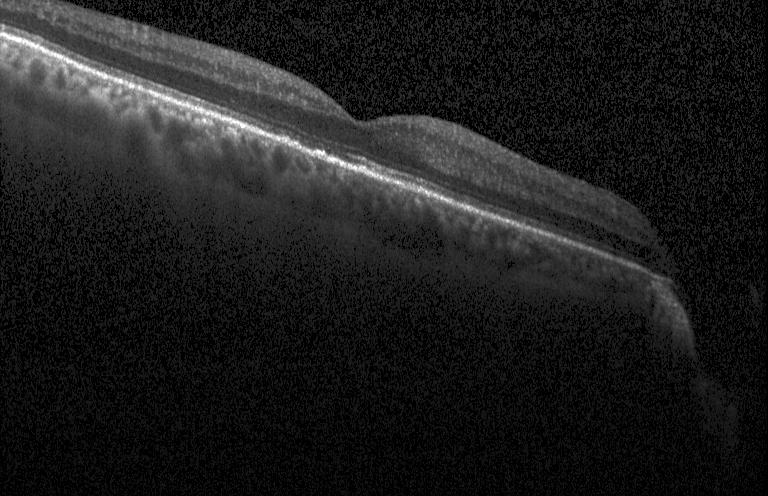 Instrument: Heidelberg Spectralis; retinal OCT B-scan.
Macular OCT: no choroidal neovascularization, no diabetic macular edema, and no drusen.